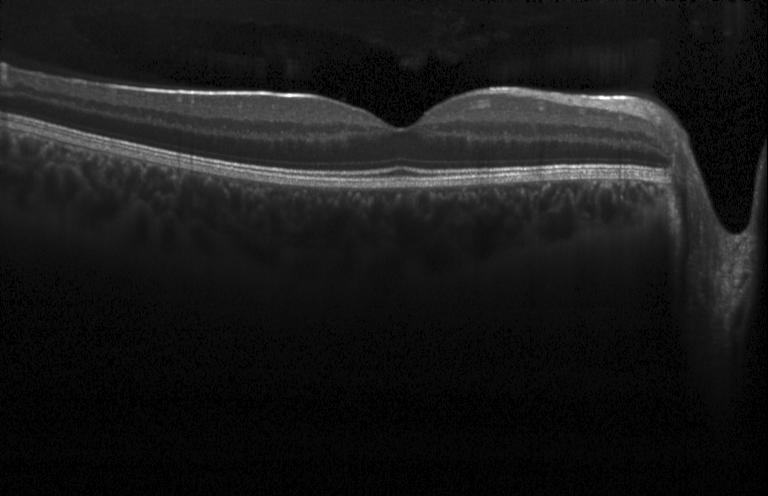 Finding: no choroidal neovascularization, diabetic macular edema, or drusen.